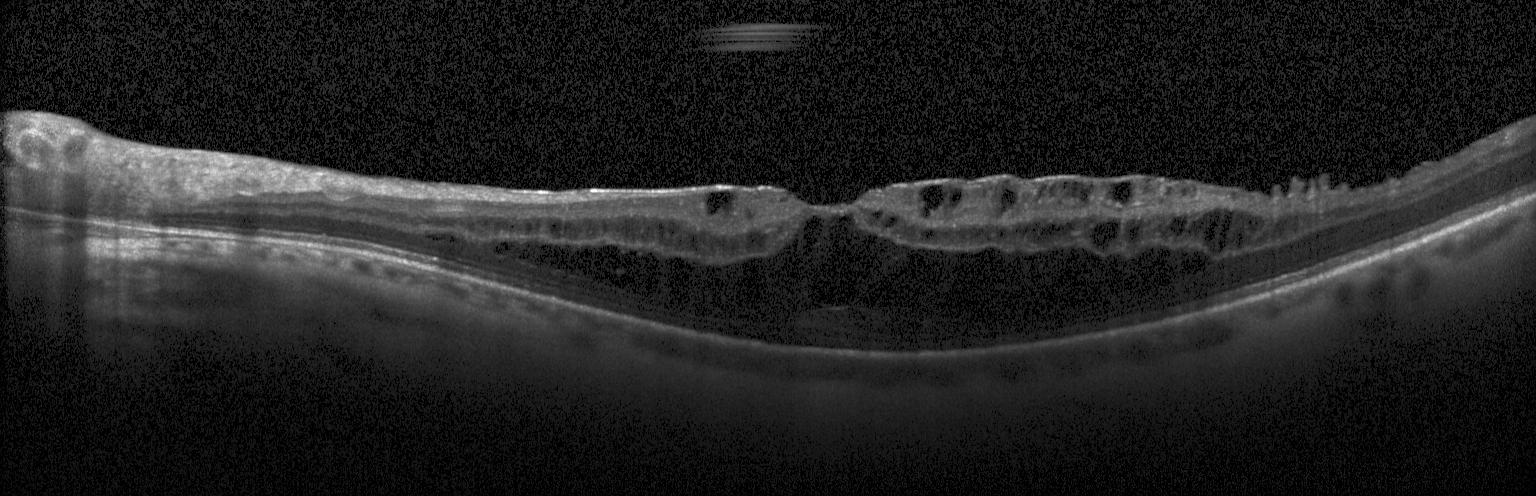

Spectral-domain OCT B-scan: diabetic macular edema.